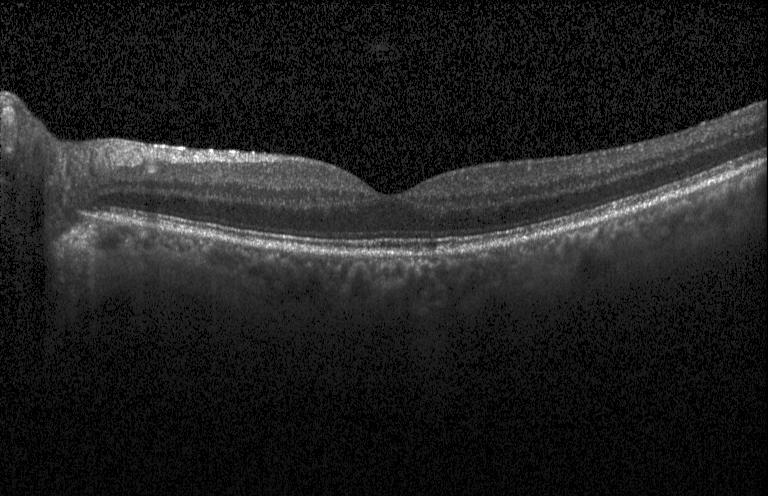

Acquired on a Heidelberg Spectralis, horizontal scan through the fovea, OCT B-scan — The scan shows no evidence of choroidal neovascularization, diabetic macular edema, or drusen.